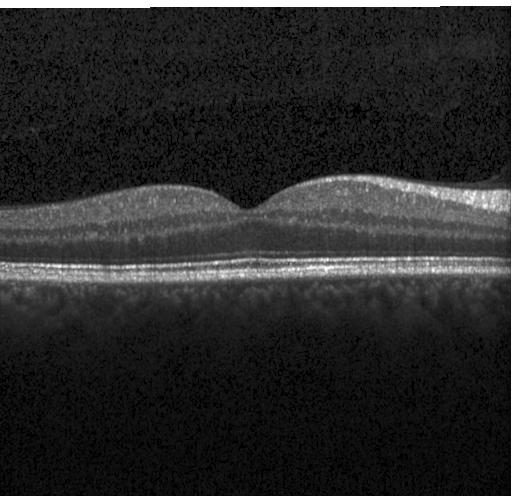 OCT finding: no evidence of CNV, DME, or drusen.